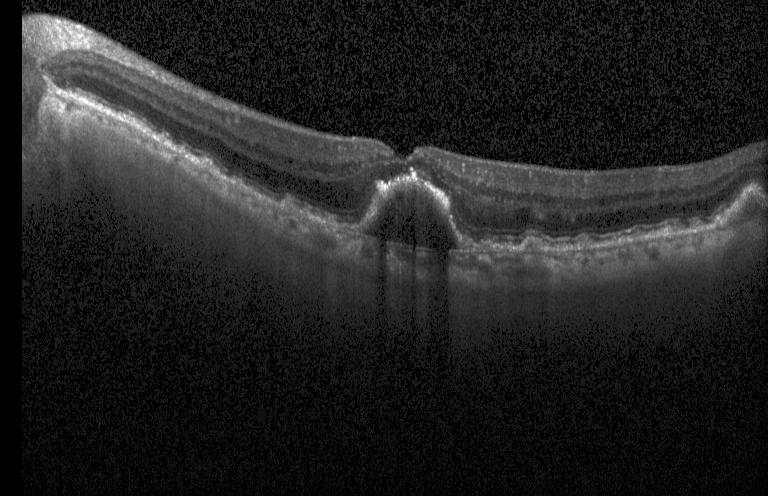

Fovea-centered; retinal OCT cross-section; spectral-domain optical coherence tomography; Heidelberg Spectralis — Diagnosis: CNV.